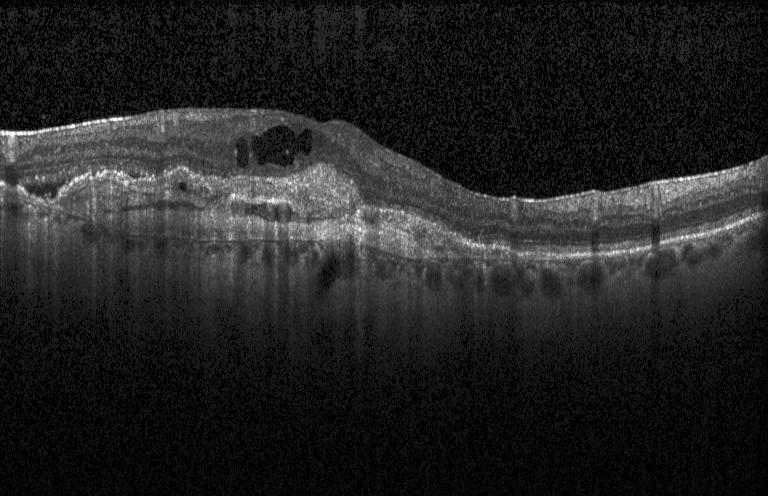
OCT B-scan. Assessment: choroidal neovascularization (CNV).